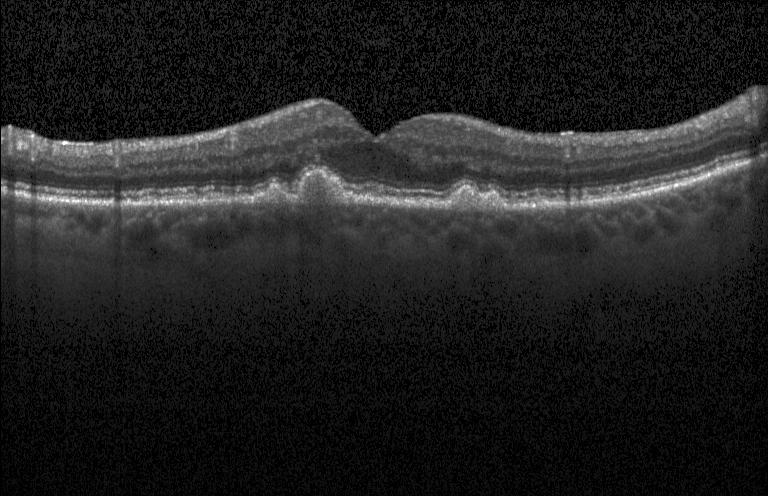
Retinal OCT cross-section
Sub-RPE drusenoid deposits.